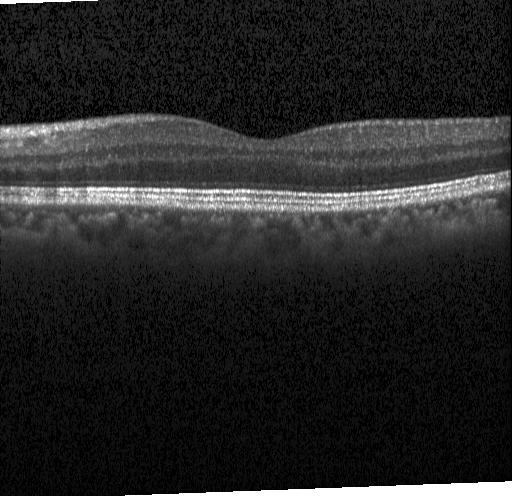
Diagnosis: neither choroidal neovascularization, diabetic macular edema, nor drusen.